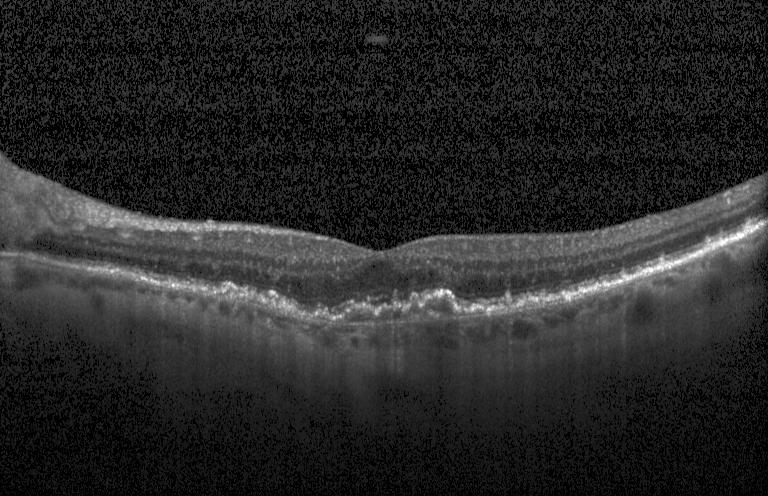

OCT finding: CNV.